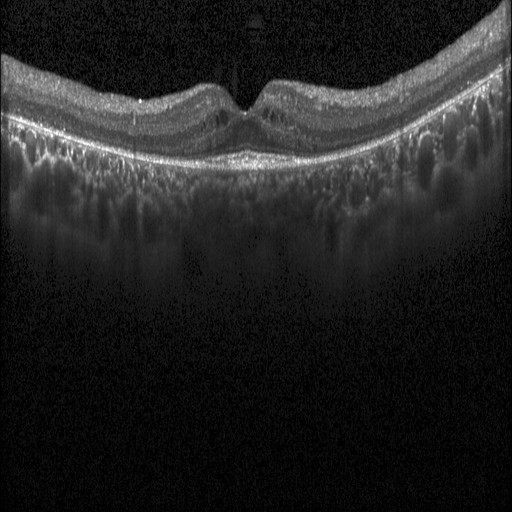 Spectral-domain OCT. Optical coherence tomography B-scan
Finding: diabetic macular edema.